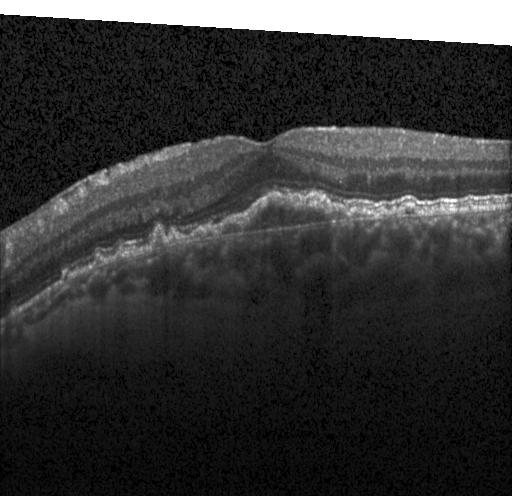
Spectral-domain OCT · instrument: Heidelberg Spectralis · optical coherence tomography scan. This B-scan demonstrates a choroidal neovascular membrane.